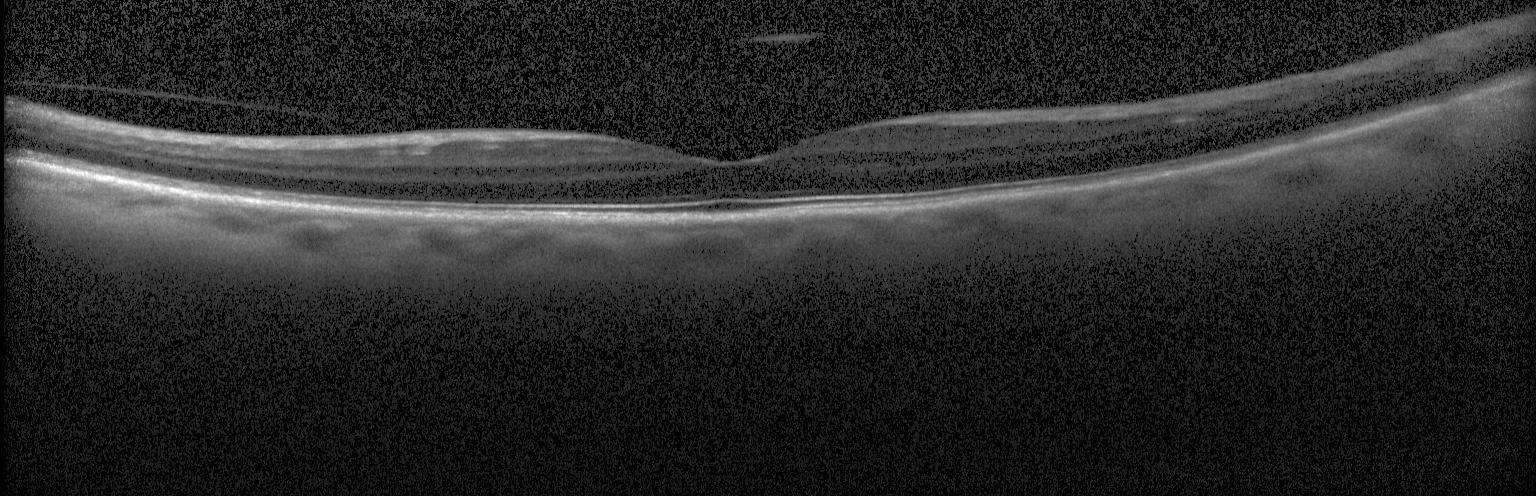
Retinal OCT B-scan. Impression: no CNV, DME, or drusen.